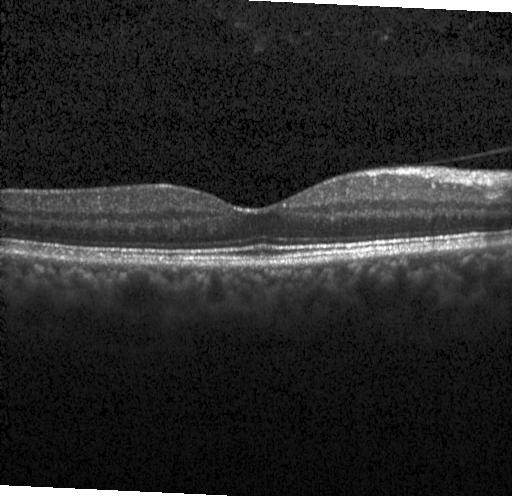 Spectral-domain OCT B-scan: neither choroidal neovascularization, diabetic macular edema, nor drusen.